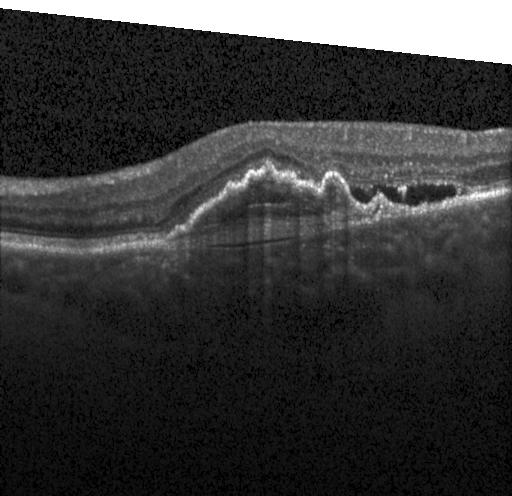
OCT scan showing a choroidal neovascular membrane.